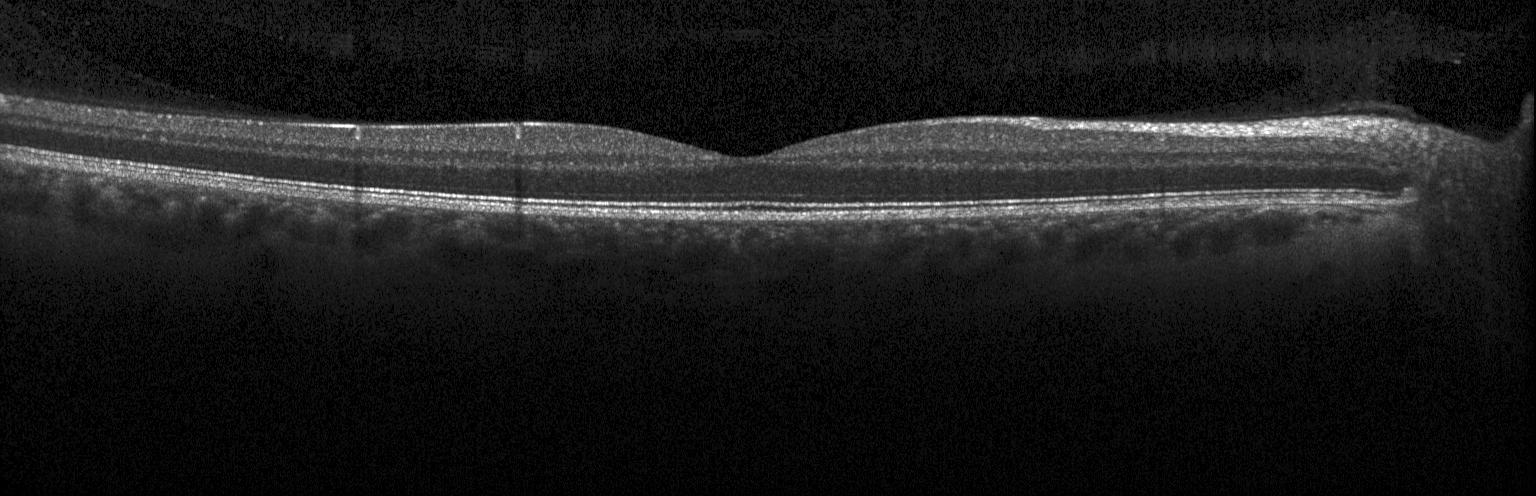 Retinal OCT B-scan · centered on the fovea · Heidelberg Spectralis OCT system · spectral-domain optical coherence tomography. This B-scan demonstrates neither CNV, DME, nor drusen.